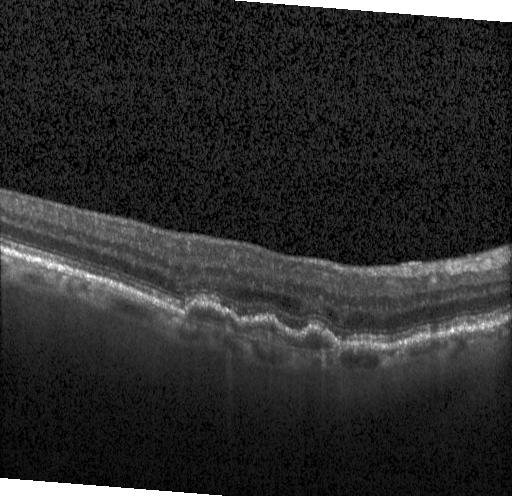
Spectral-domain optical coherence tomography. Retinal OCT cross-section. Diagnosis: CNV.